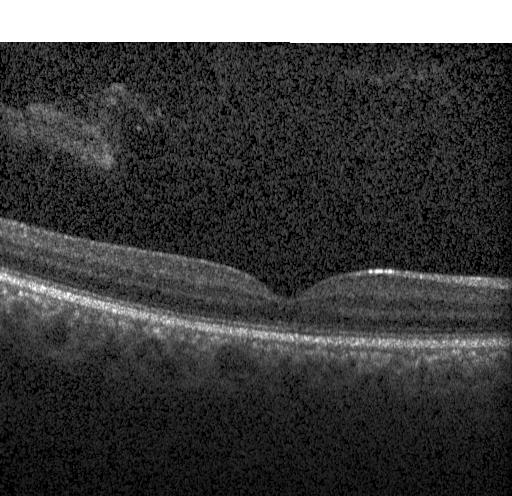
OCT finding: no choroidal neovascularization, diabetic macular edema, or drusen.